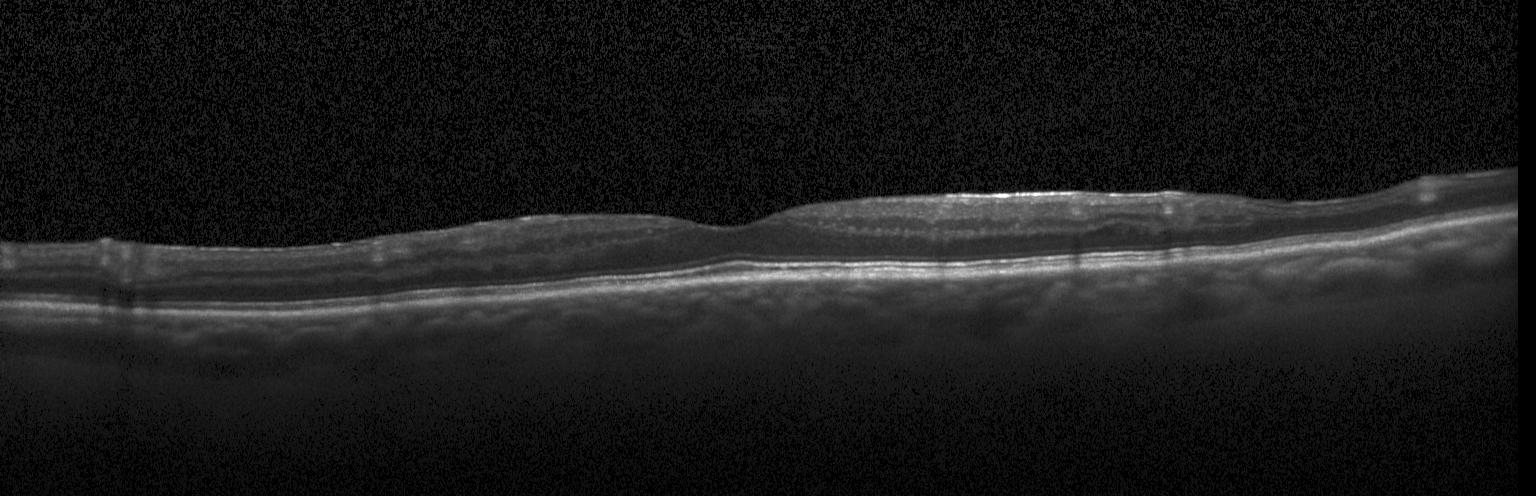
Impression: no CNV, DME, or drusen.